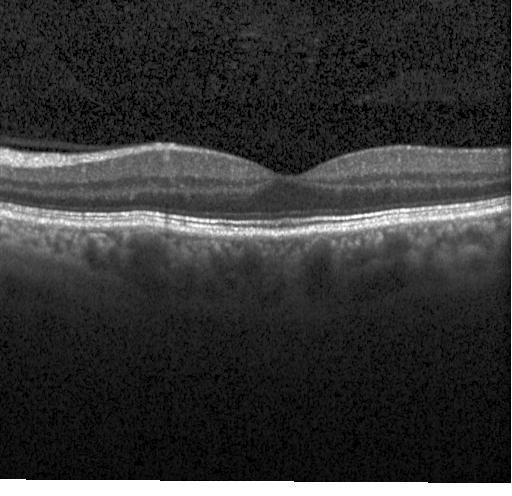

OCT B-scan. Macular scan.
Neither CNV, DME, nor drusen.